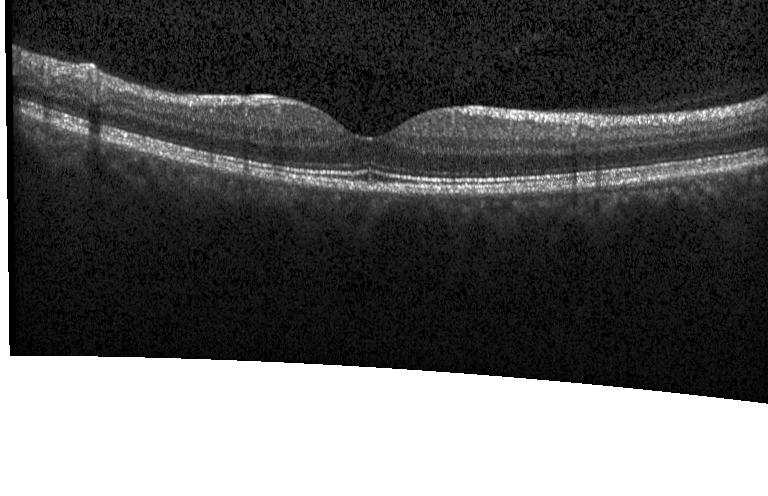
OCT B-scan · Heidelberg Spectralis OCT system. Impression: neither choroidal neovascularization, diabetic macular edema, nor drusen.